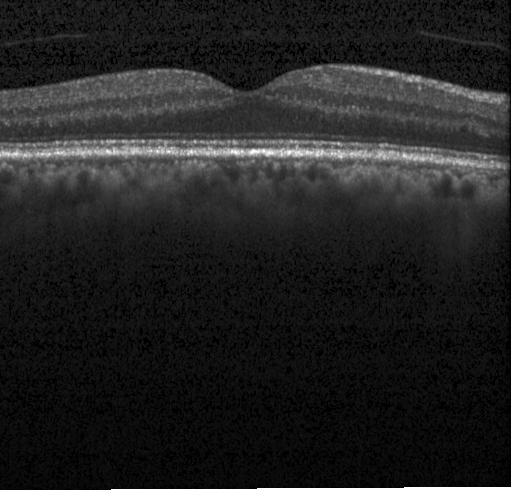

OCT line scan.
Diagnosis: neither CNV, DME, nor drusen.